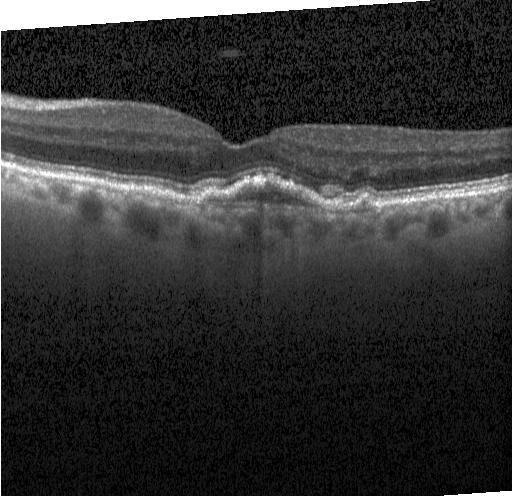

Acquired on a Heidelberg Spectralis, SD-OCT, optical coherence tomography scan, horizontal scan through the fovea.
Macular OCT: a choroidal neovascular membrane.